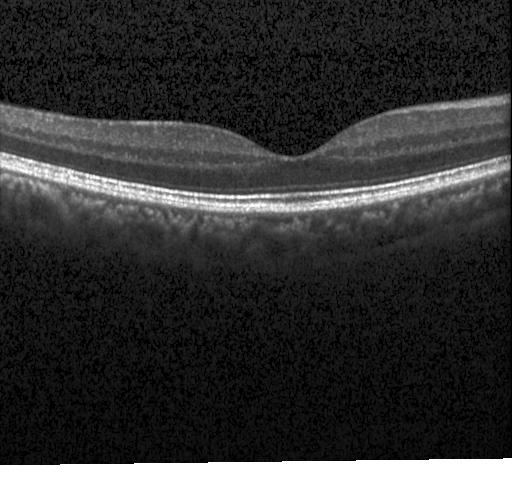
Dx: no choroidal neovascularization, diabetic macular edema, or drusen.